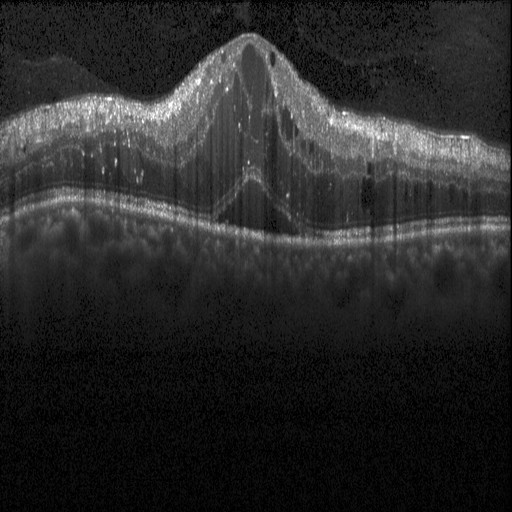
OCT B-scan. This B-scan demonstrates DME.